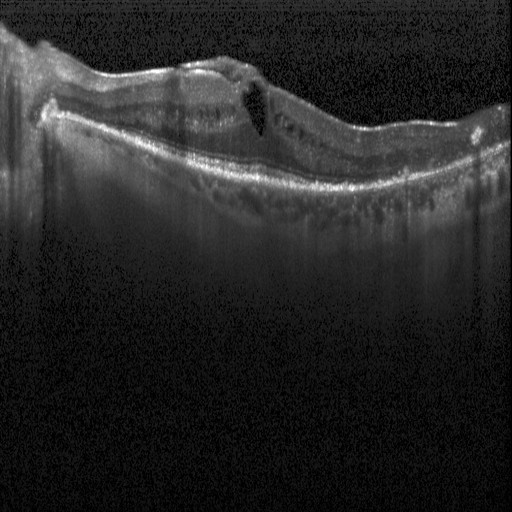 Retinal OCT B-scan — Diagnosis: DME.